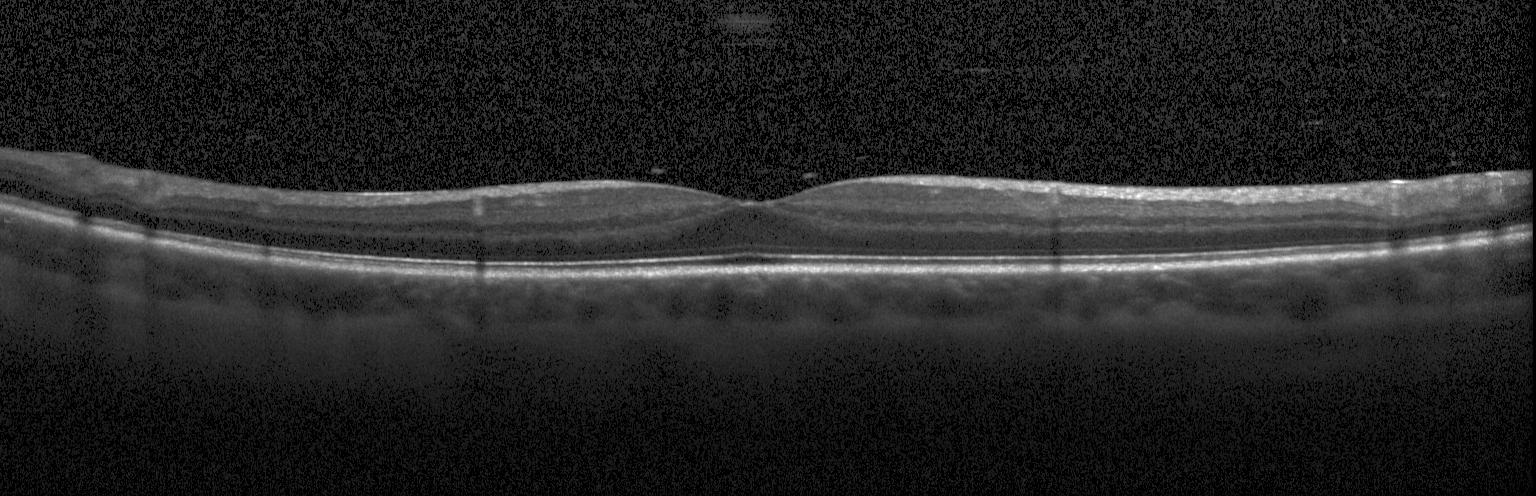

Dx: no choroidal neovascularization, no diabetic macular edema, and no drusen.